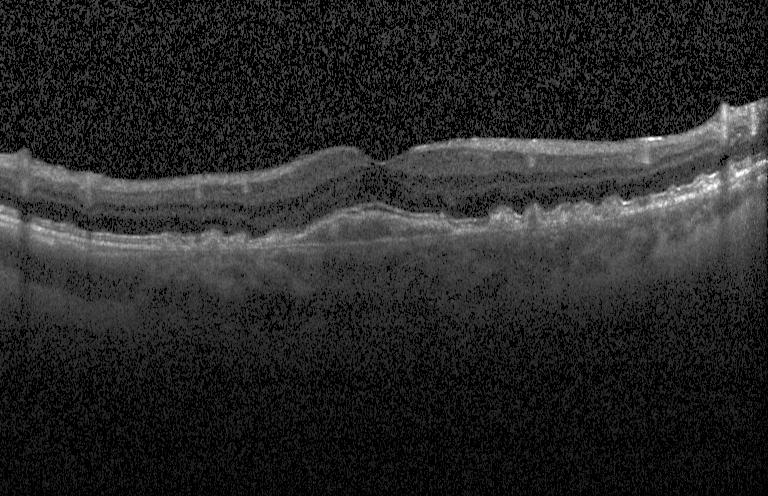
This B-scan demonstrates a choroidal neovascular membrane.